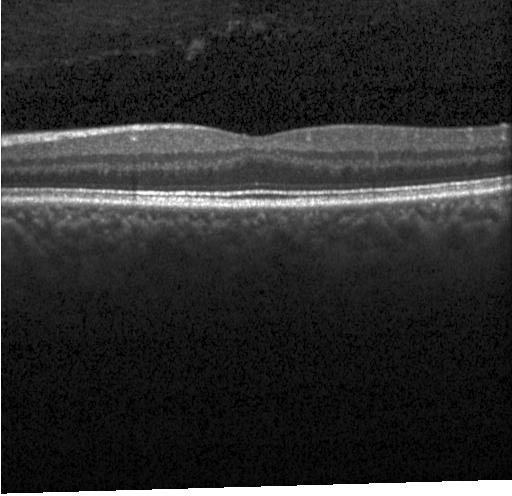

Instrument: Heidelberg Spectralis · SD-OCT · retinal OCT cross-section · fovea-centered.
Impression: no choroidal neovascularization, no diabetic macular edema, and no drusen.